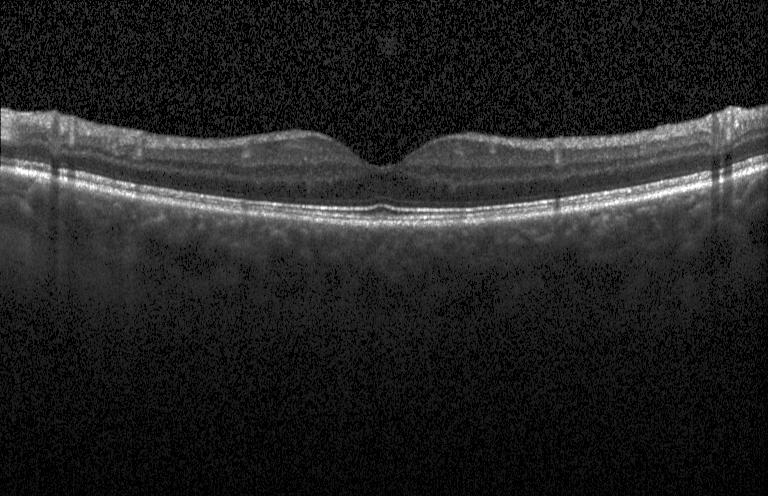

Acquired on a Heidelberg Spectralis, retinal OCT B-scan, fovea-centered, spectral-domain optical coherence tomography — Diagnosis: no evidence of CNV, DME, or drusen.